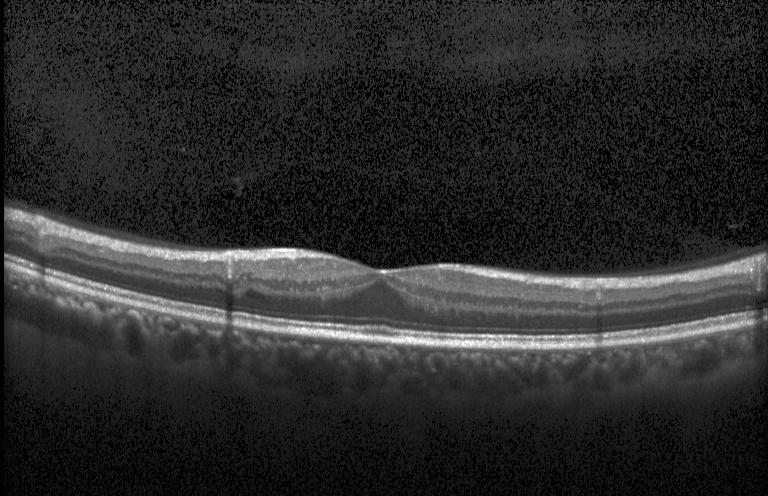 OCT finding: no choroidal neovascularization, no diabetic macular edema, and no drusen.